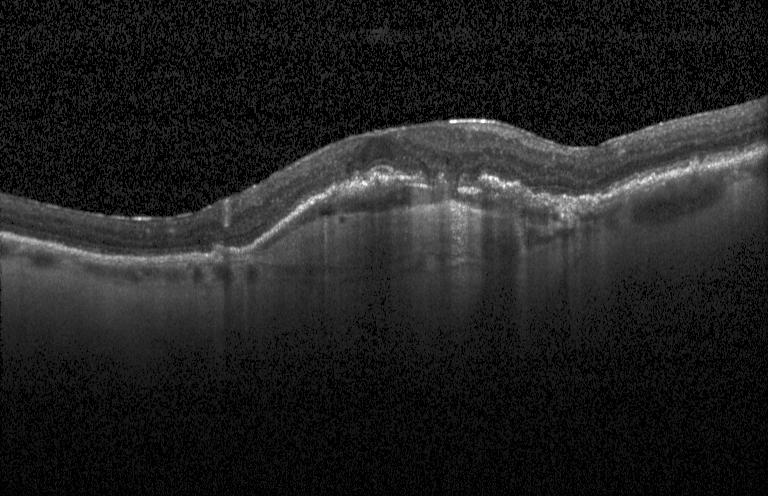 Macular scan; optical coherence tomography scan.
This B-scan demonstrates a choroidal neovascular membrane.